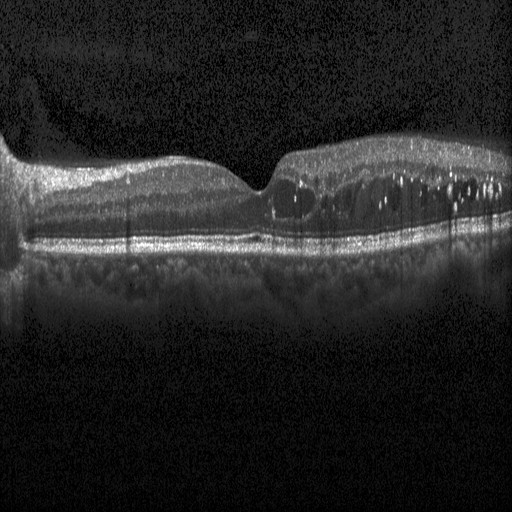

Instrument: Heidelberg Spectralis. Centered on the fovea. Optical coherence tomography B-scan. SD-OCT.
Assessment: DME.